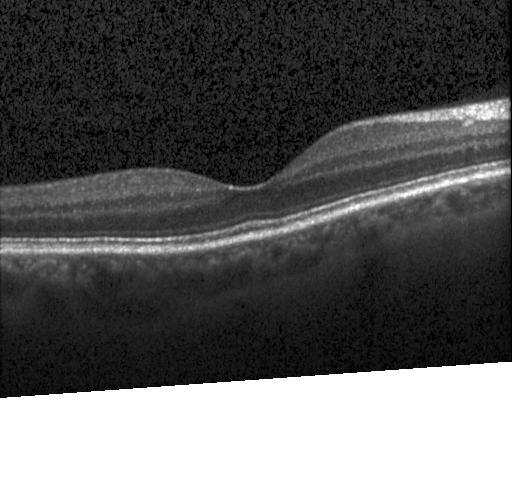

OCT scan showing no choroidal neovascularization, diabetic macular edema, or drusen.